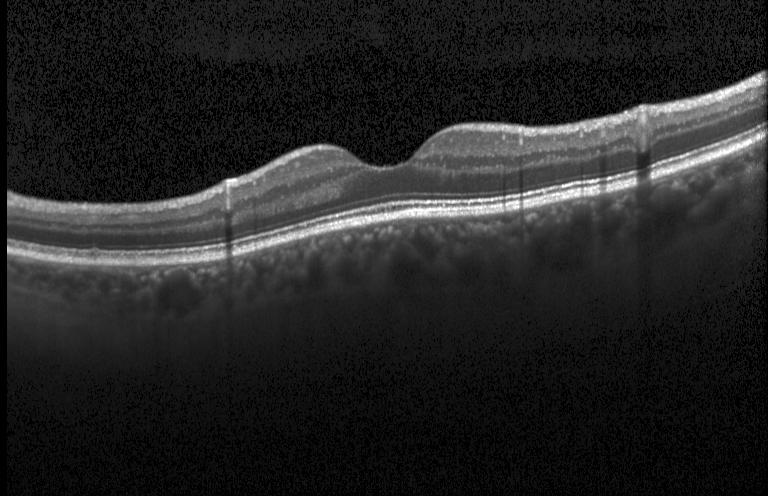
Impression: no choroidal neovascularization, no diabetic macular edema, and no drusen.